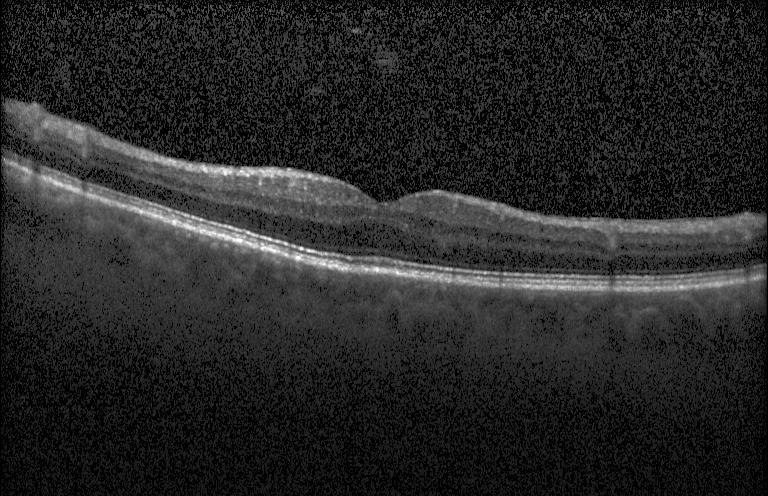
The scan shows no choroidal neovascularization, diabetic macular edema, or drusen.